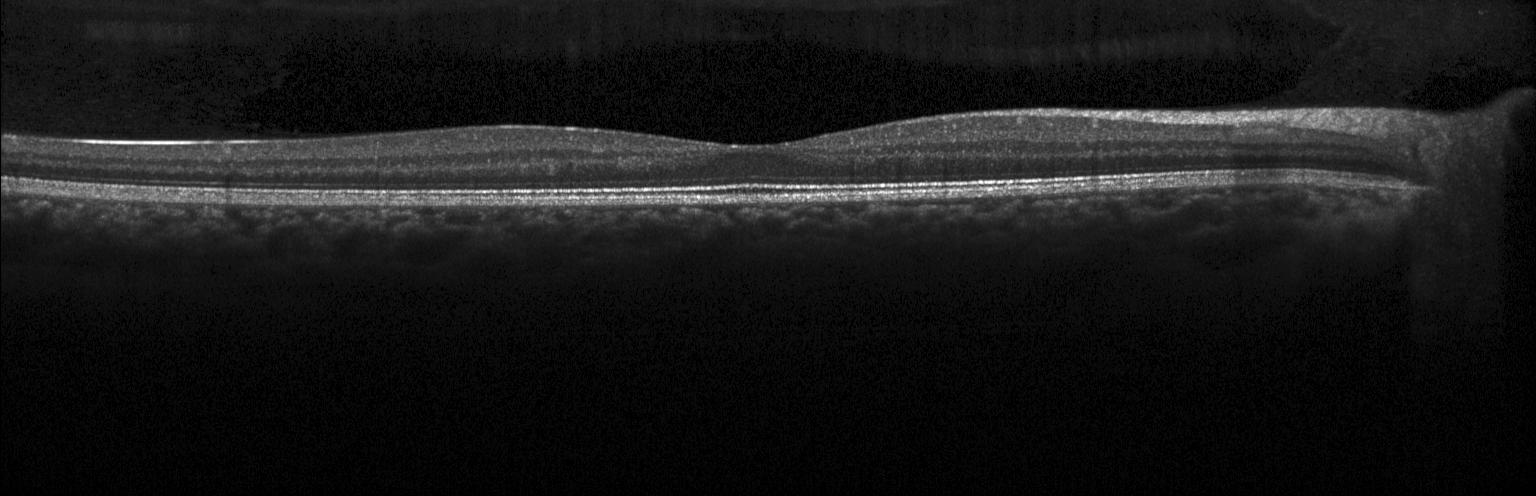

SD-OCT, instrument: Heidelberg Spectralis, OCT B-scan, macular scan — Diagnosis: no choroidal neovascularization, no diabetic macular edema, and no drusen.